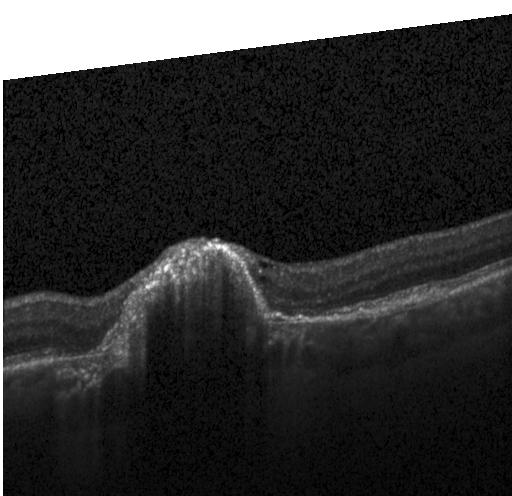 Spectral-domain OCT B-scan: choroidal neovascularization (CNV).